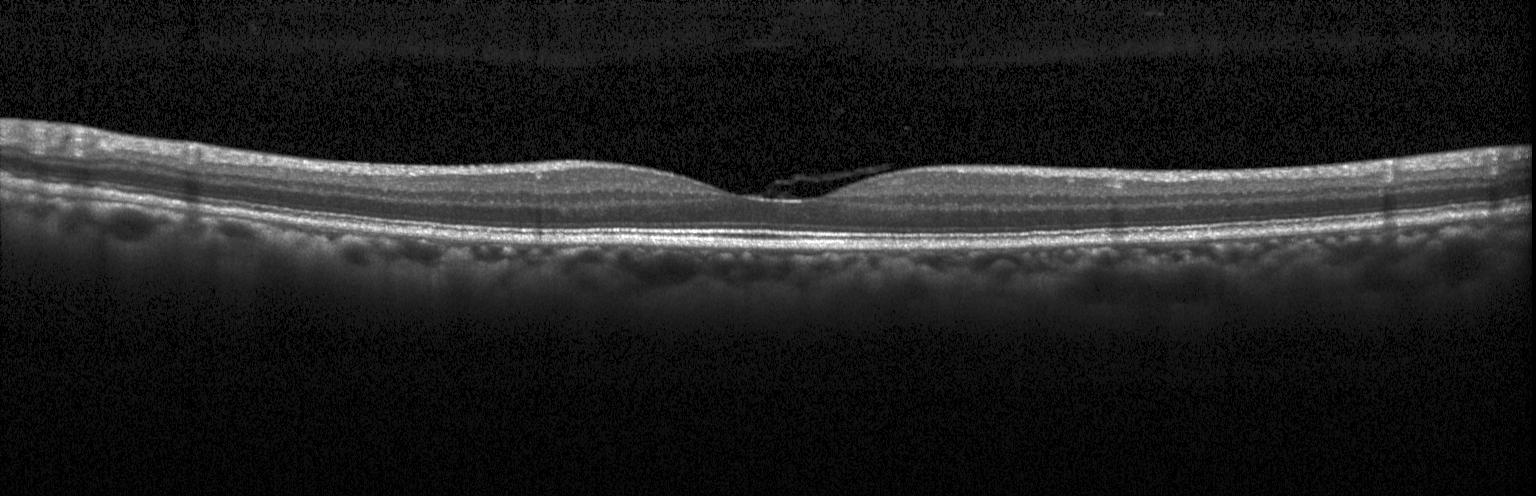
Through the macula, retinal OCT B-scan, instrument: Heidelberg Spectralis, spectral-domain optical coherence tomography. Dx: neither choroidal neovascularization, diabetic macular edema, nor drusen.